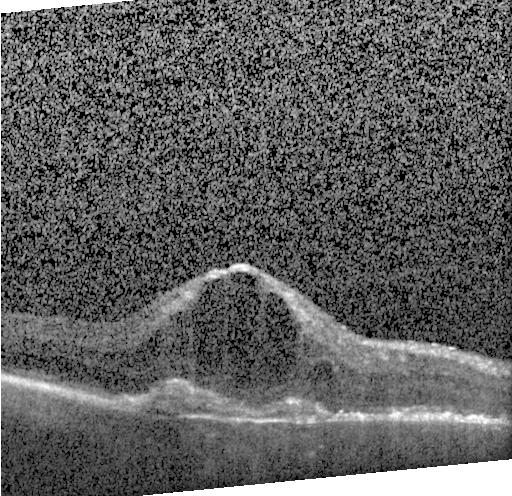
Finding: a choroidal neovascular membrane.